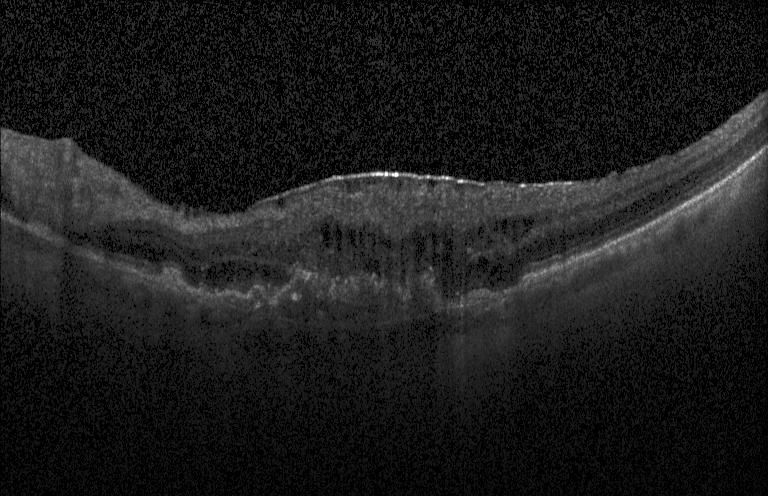 Optical coherence tomography scan.
OCT finding: a choroidal neovascular membrane.